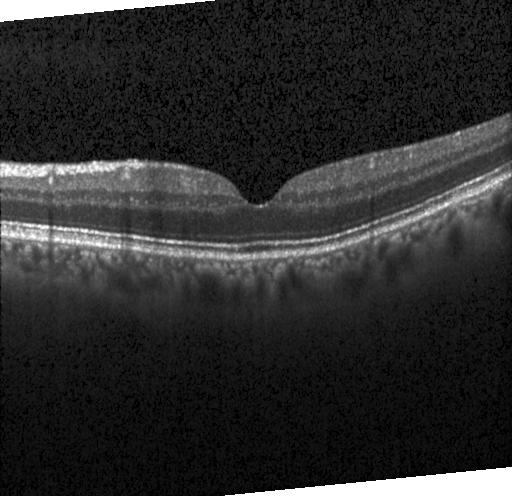 OCT B-scan. Impression: no choroidal neovascularization, no diabetic macular edema, and no drusen.